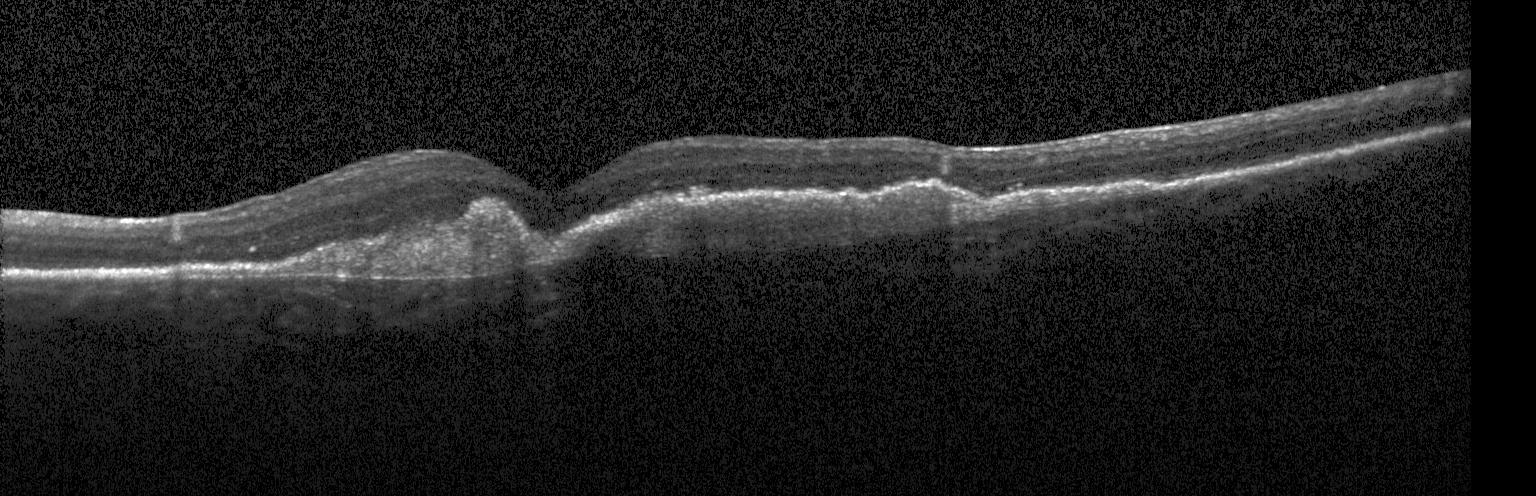 Optical coherence tomography B-scan, centered on the fovea, SD-OCT, acquired on a Heidelberg Spectralis. Finding: a choroidal neovascular membrane.